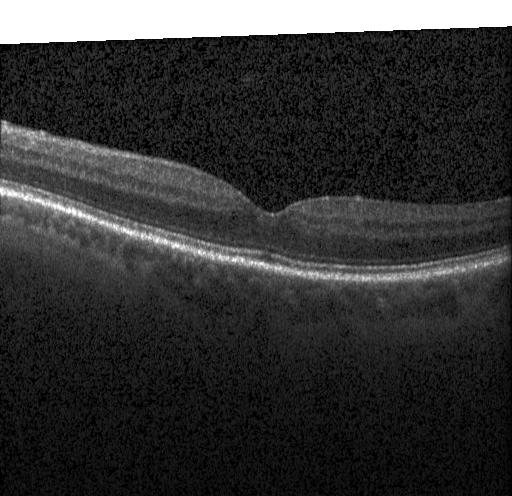
Retinal OCT B-scan. Diagnosis: no evidence of choroidal neovascularization, diabetic macular edema, or drusen.